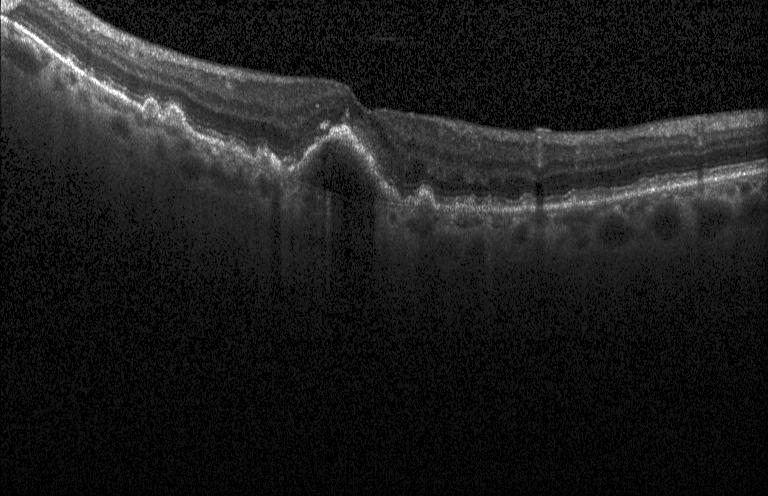 Acquired on a Heidelberg Spectralis; OCT B-scan
Dx: choroidal neovascularization (CNV).